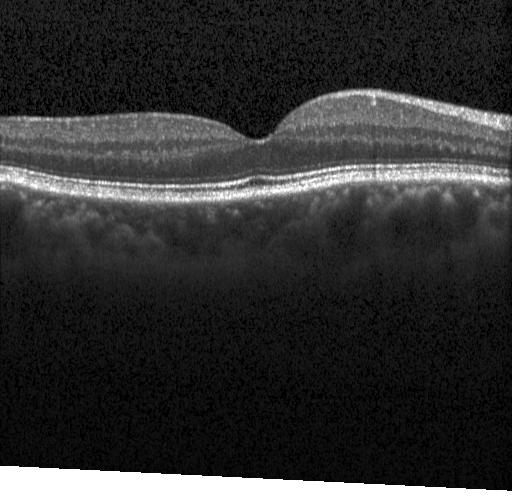
Retinal OCT B-scan. The scan shows no evidence of CNV, DME, or drusen.